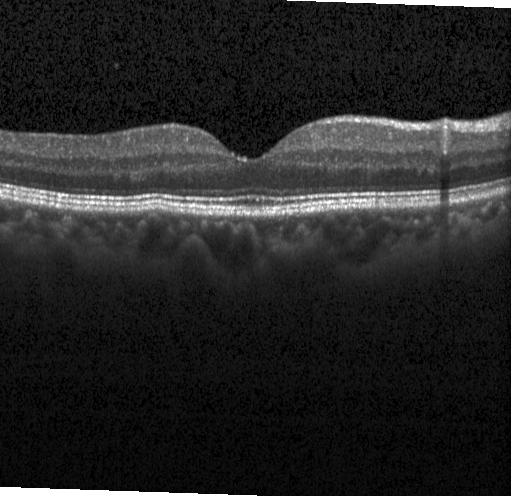
Macular scan, spectral-domain OCT, retinal OCT cross-section — Assessment: no CNV, no DME, and no drusen.